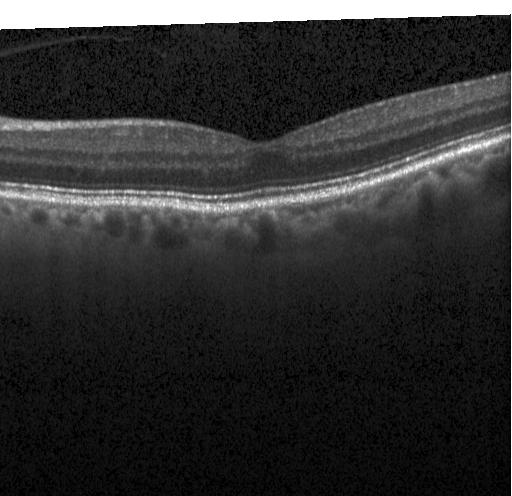
Spectral-domain OCT. Fovea-centered. OCT B-scan. Instrument: Heidelberg Spectralis. Impression: no CNV, no DME, and no drusen.